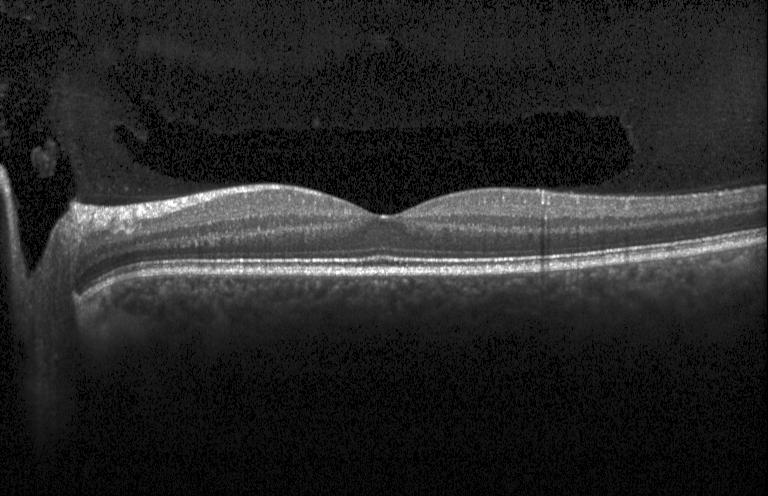
Macular scan, retinal OCT B-scan
Finding: no choroidal neovascularization, diabetic macular edema, or drusen.